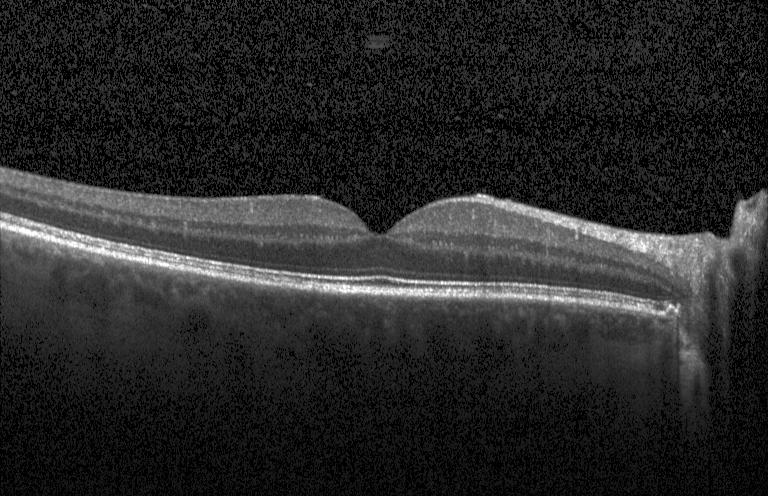 Acquired on a Heidelberg Spectralis; SD-OCT; optical coherence tomography B-scan; macular scan
This B-scan demonstrates neither choroidal neovascularization, diabetic macular edema, nor drusen.